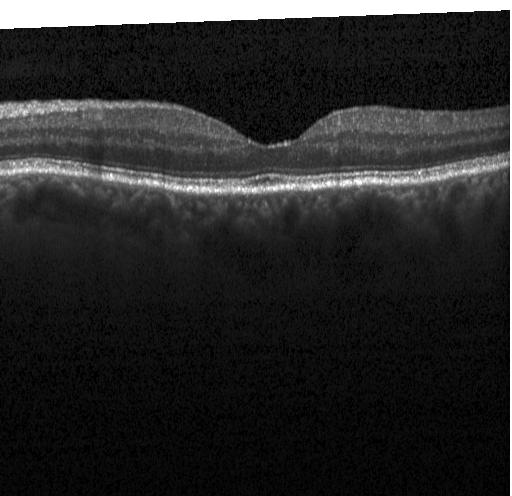
Neither CNV, DME, nor drusen.